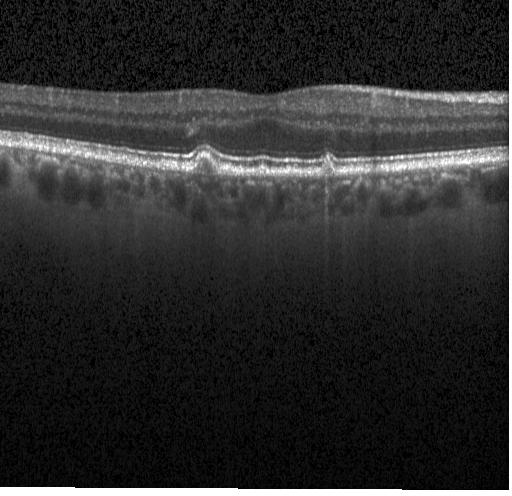 OCT finding: sub-RPE drusenoid deposits.